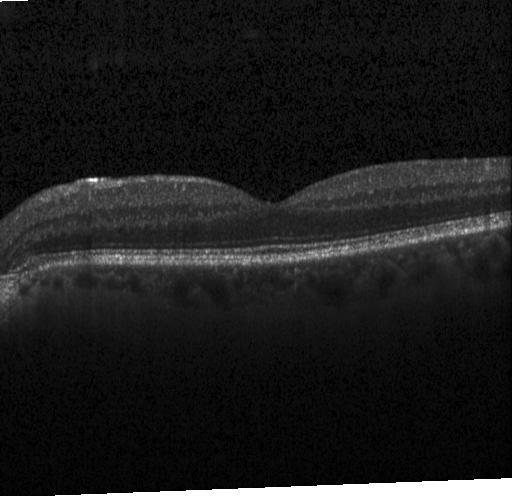

Macular OCT: no choroidal neovascularization, no diabetic macular edema, and no drusen.